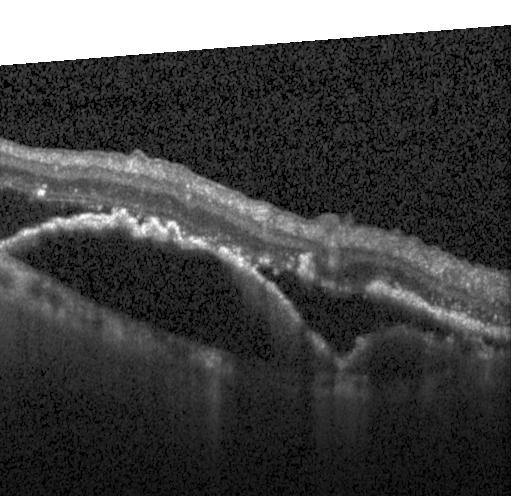
Retinal OCT B-scan.
Finding: a choroidal neovascular membrane.